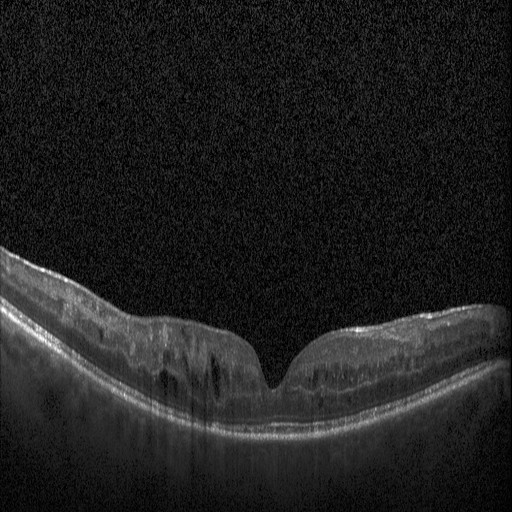

SD-OCT; horizontal scan through the fovea; OCT line scan.
Assessment: DME.